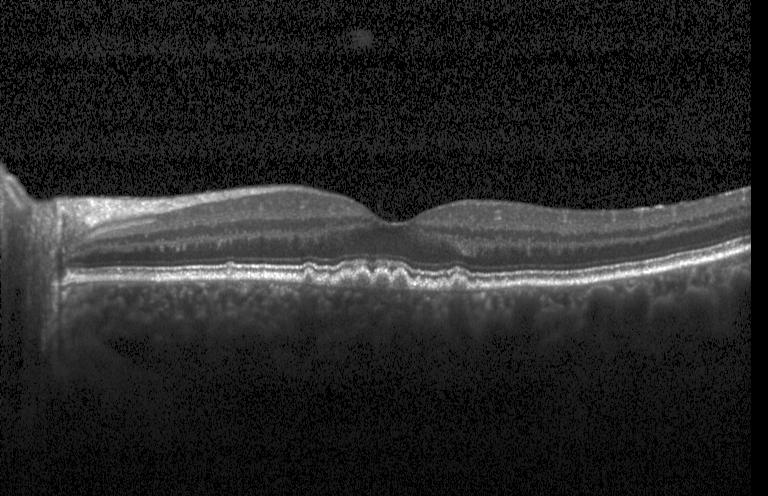

Macular OCT demonstrating sub-RPE drusenoid deposits.